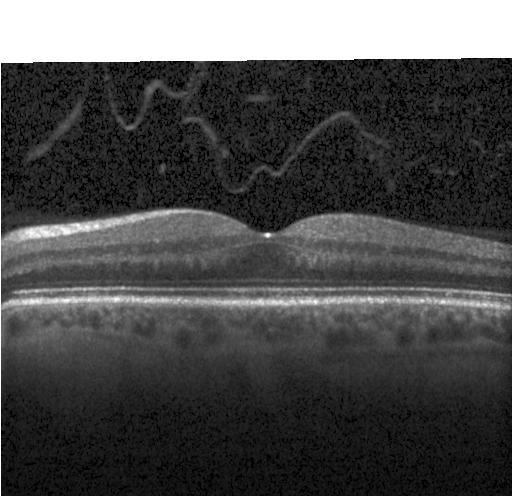
Optical coherence tomography B-scan. Through the macula. Acquired on a Heidelberg Spectralis — Diagnosis: no choroidal neovascularization, diabetic macular edema, or drusen.